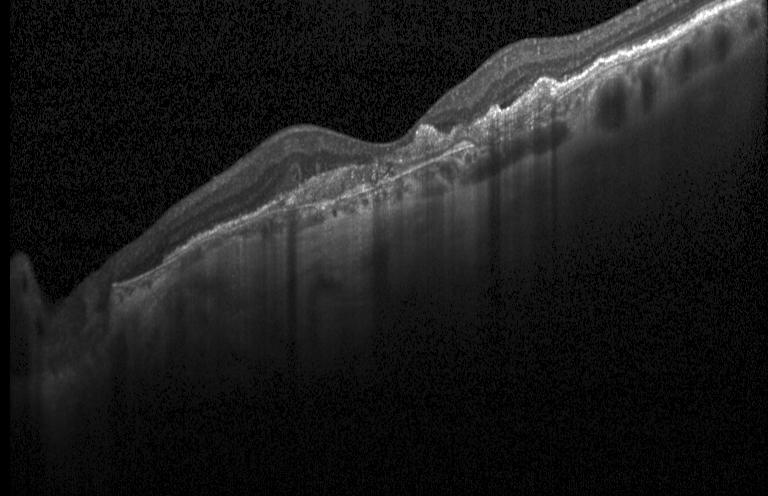 OCT finding: a choroidal neovascular membrane.